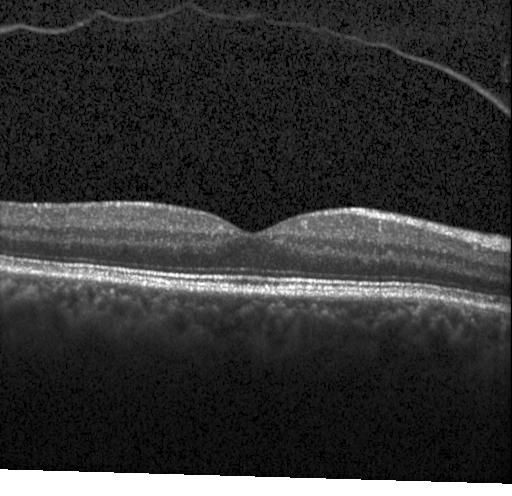 Finding: neither CNV, DME, nor drusen.